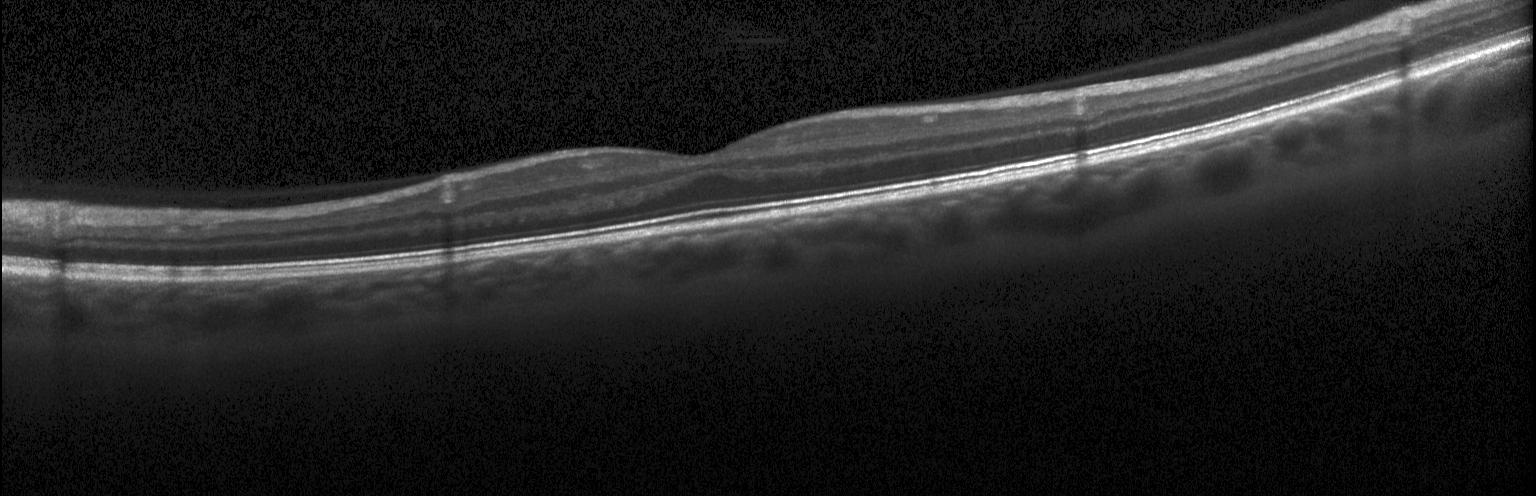

Horizontal scan through the fovea. Retinal OCT cross-section. Heidelberg Spectralis OCT system.
The scan shows no CNV, no DME, and no drusen.